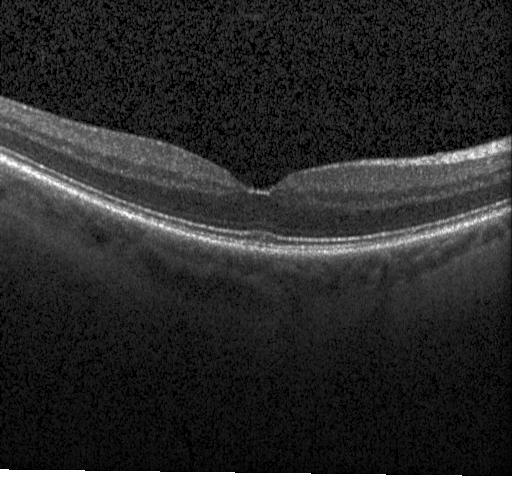
Dx: no choroidal neovascularization, diabetic macular edema, or drusen.